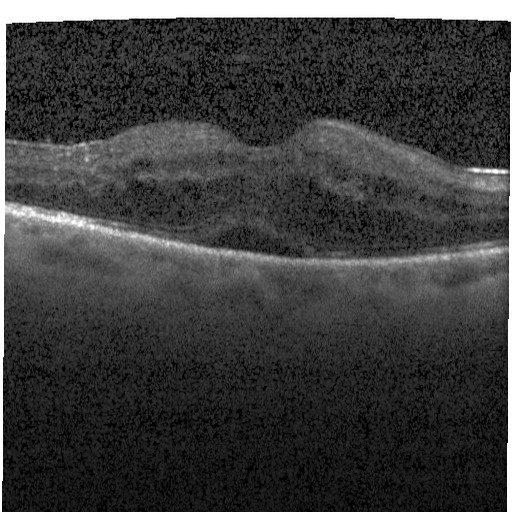
Macular OCT demonstrating diabetic macular edema (DME).